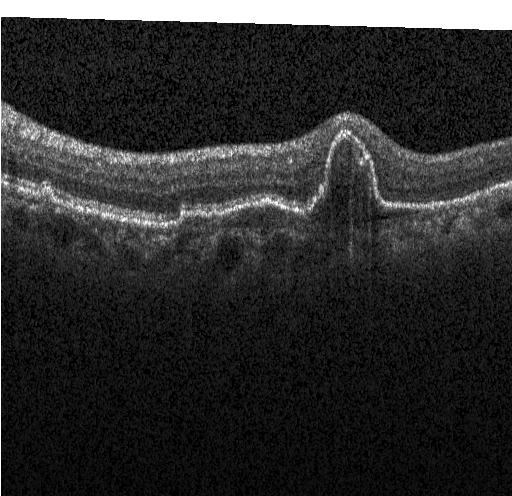

OCT line scan.
The scan shows choroidal neovascularization.